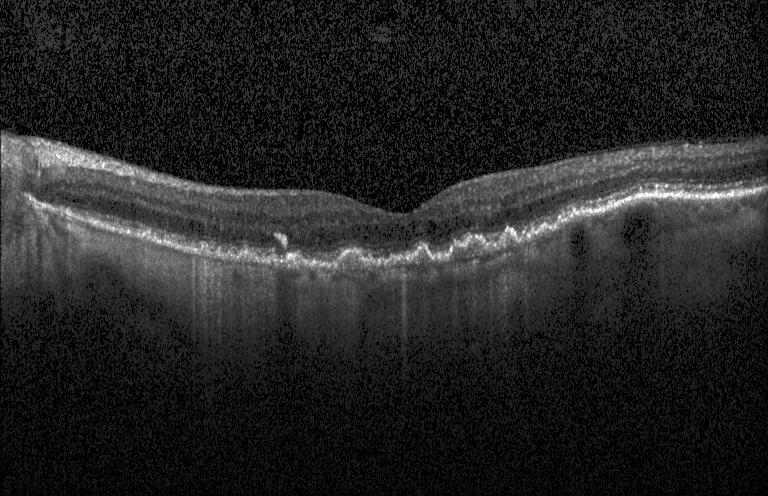
Retinal OCT cross-section — Diagnosis: a choroidal neovascular membrane.